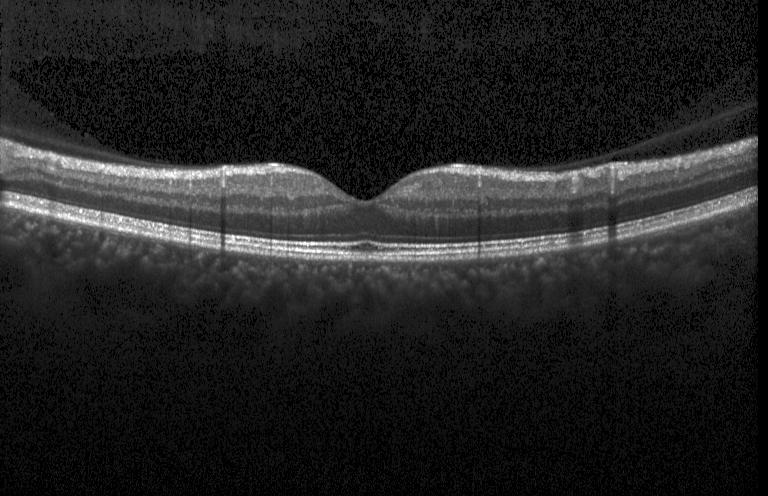
Finding: no CNV, no DME, and no drusen.